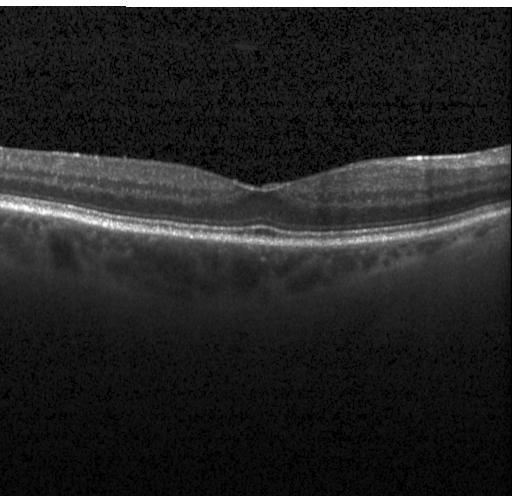 Acquired on a Heidelberg Spectralis. OCT B-scan. Spectral-domain optical coherence tomography
Diagnosis: no evidence of choroidal neovascularization, diabetic macular edema, or drusen.